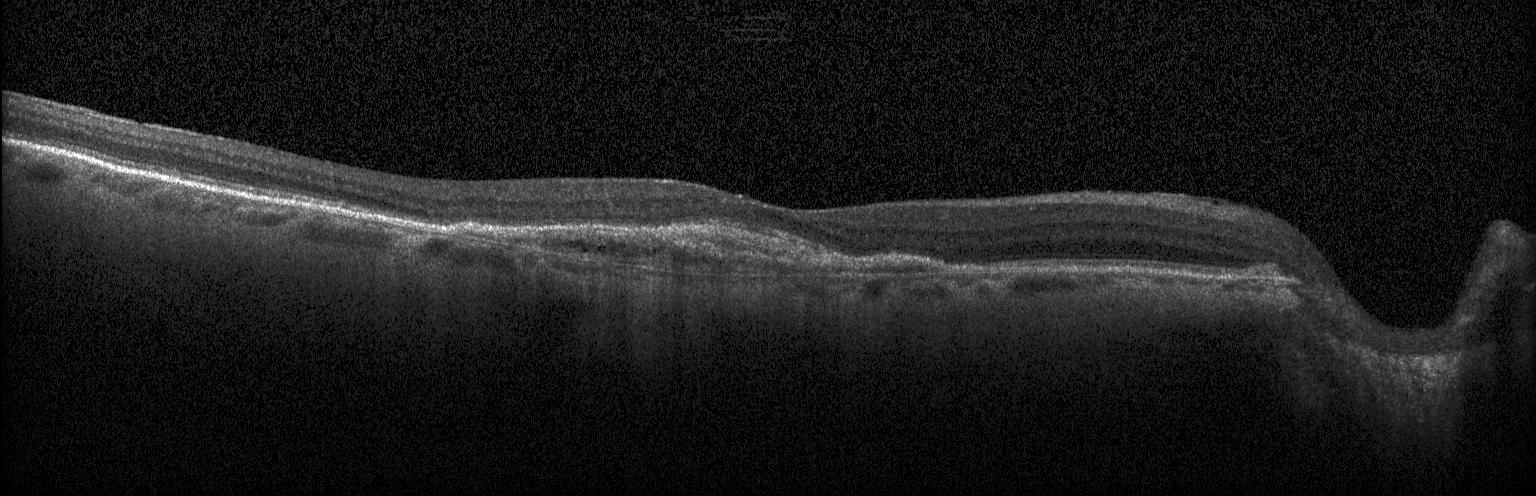
OCT line scan. Impression: choroidal neovascularization.